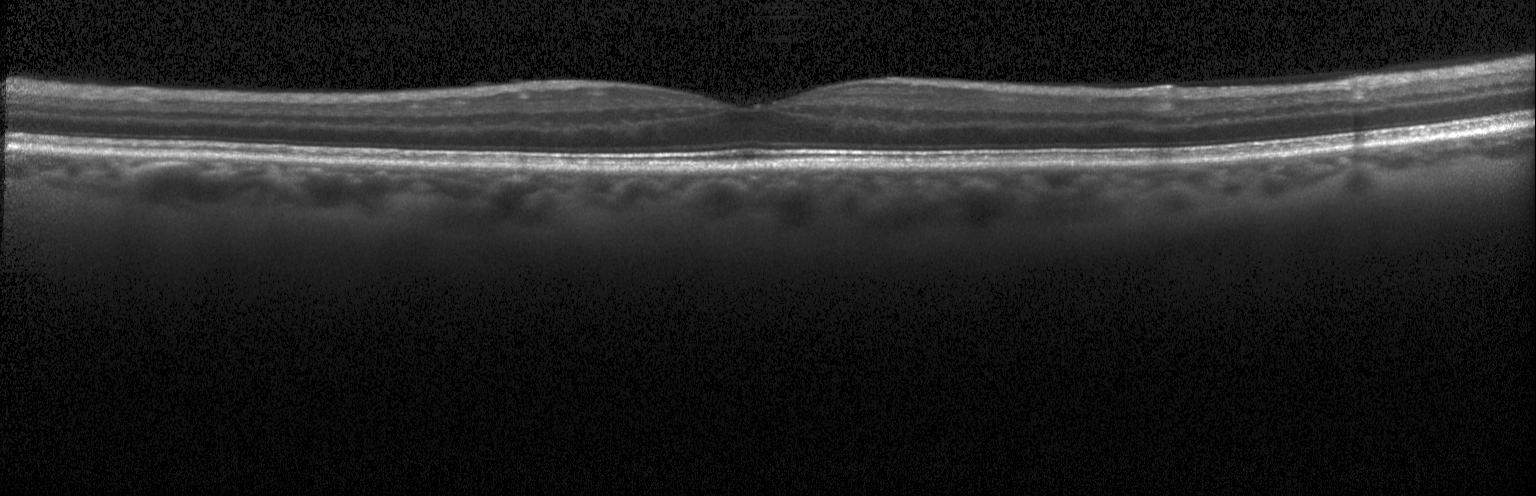
Finding: no evidence of choroidal neovascularization, diabetic macular edema, or drusen.